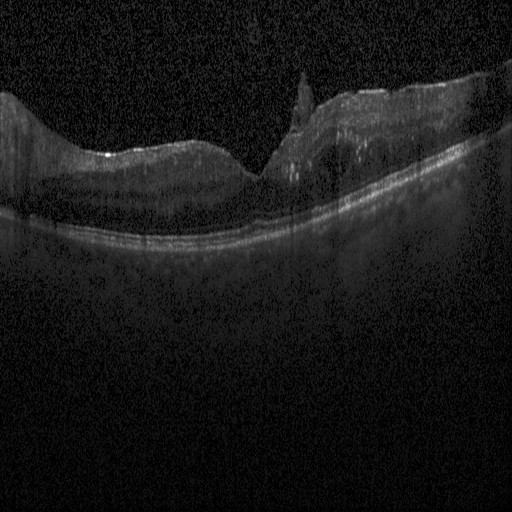
Optical coherence tomography scan; spectral-domain OCT; horizontal scan through the fovea; Heidelberg Spectralis. Diagnosis: diabetic macular edema (DME).